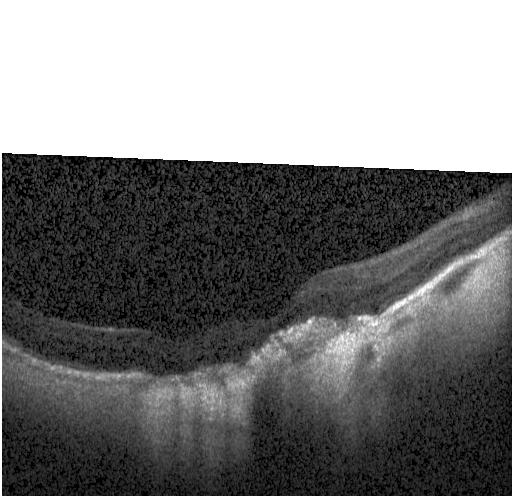

Retinal OCT cross-section
OCT finding: a choroidal neovascular membrane.